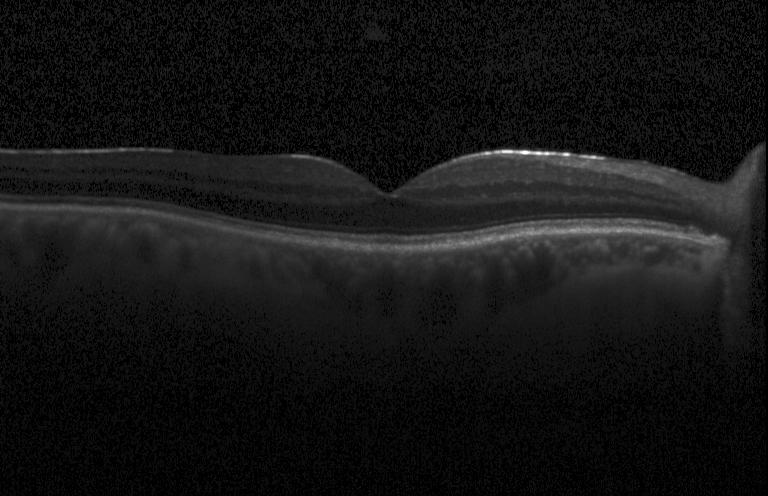 Optical coherence tomography B-scan. Spectral-domain OCT. Acquired on a Heidelberg Spectralis. Fovea-centered. Finding: no evidence of choroidal neovascularization, diabetic macular edema, or drusen.